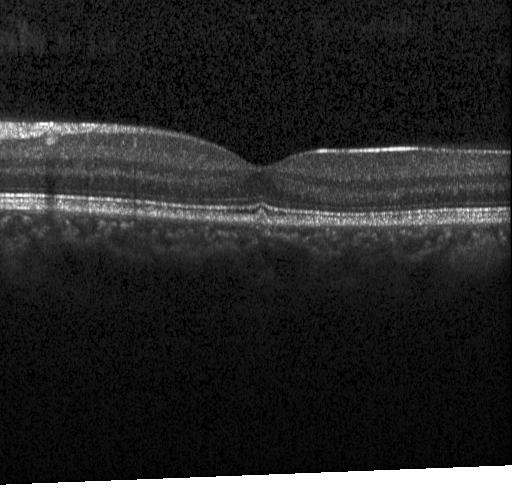

OCT line scan. Centered on the fovea
Impression: sub-RPE drusenoid deposits.